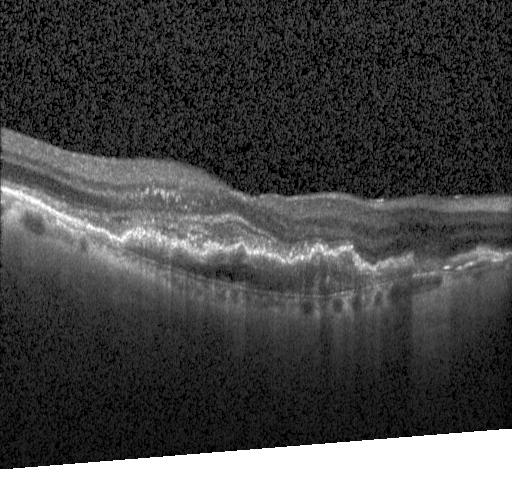 Heidelberg Spectralis · macular scan · SD-OCT · optical coherence tomography B-scan — Diagnosis: choroidal neovascularization.